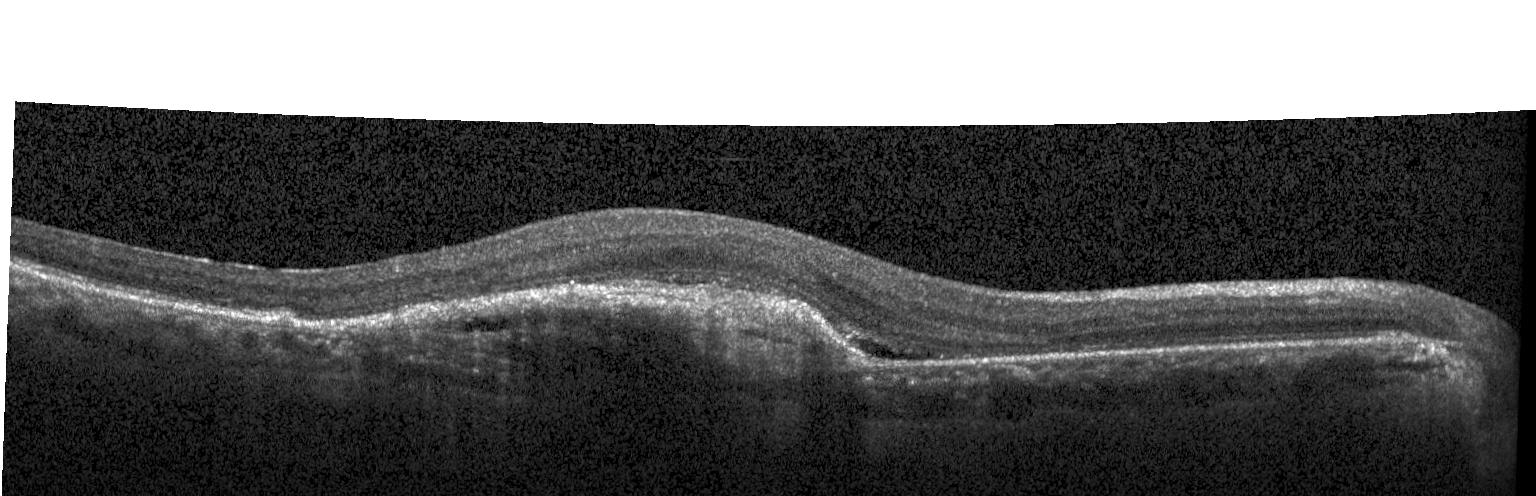

OCT line scan; spectral-domain OCT; Heidelberg Spectralis OCT system.
Choroidal neovascularization.